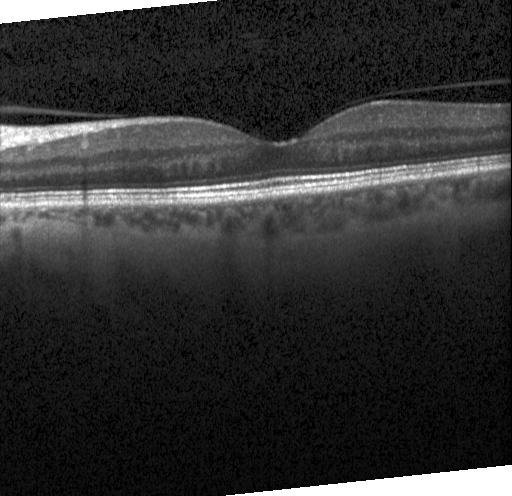

OCT line scan — No choroidal neovascularization, diabetic macular edema, or drusen.